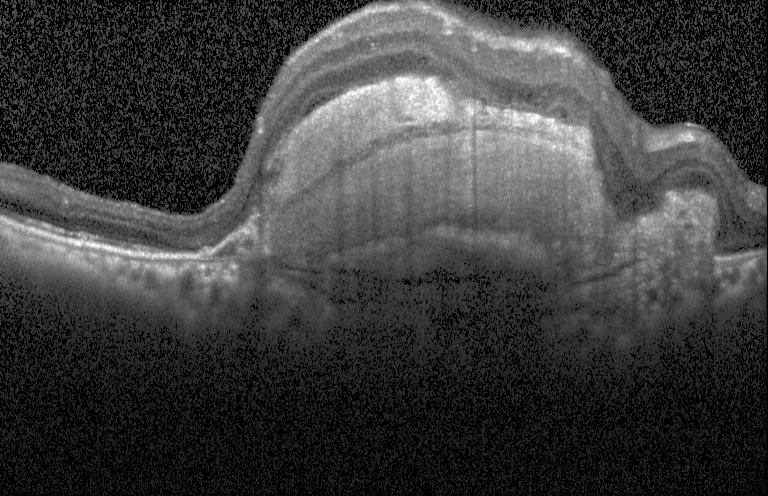 Spectral-domain OCT B-scan: choroidal neovascularization.